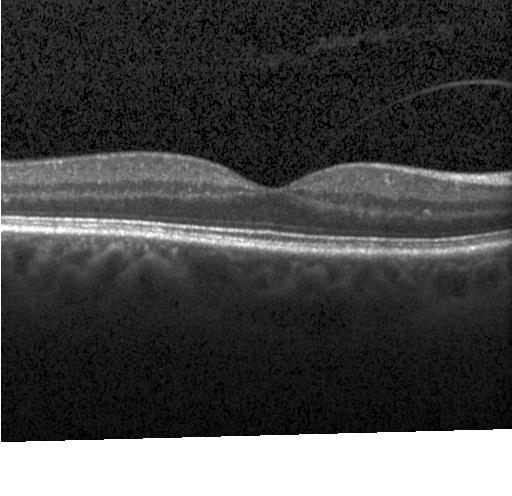 Retinal OCT cross-section. Heidelberg Spectralis. Horizontal scan through the fovea. SD-OCT — Diagnosis: no choroidal neovascularization, diabetic macular edema, or drusen.